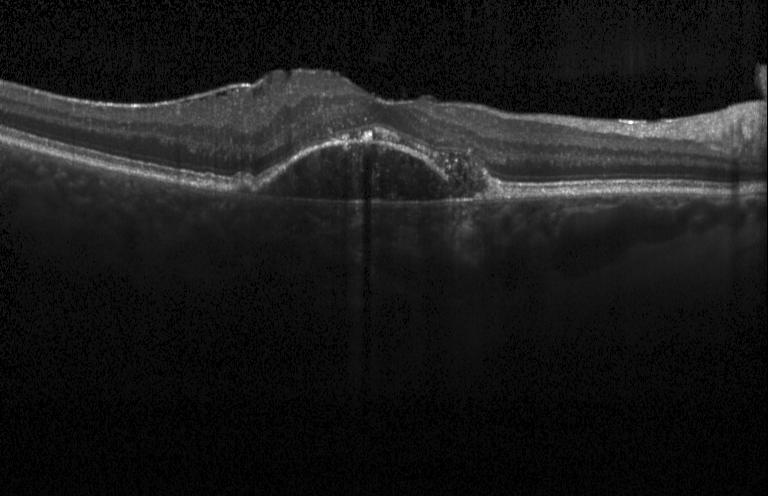
Macular OCT demonstrating a choroidal neovascular membrane.